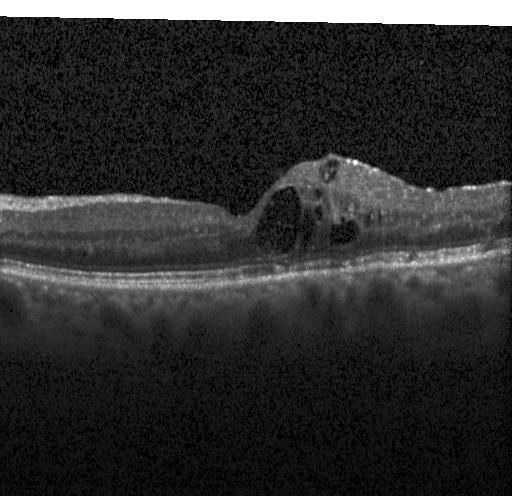 OCT finding: diabetic macular edema (DME).